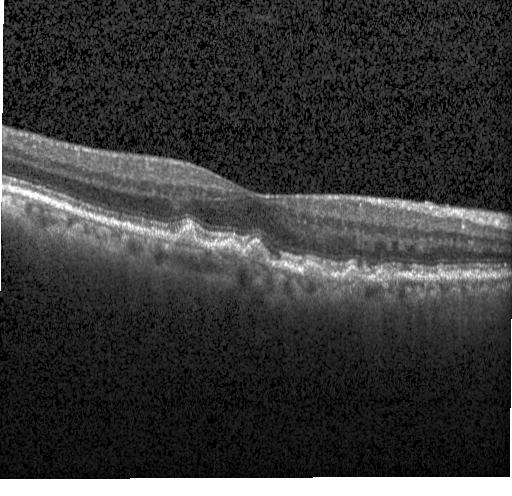 Impression: drusen.